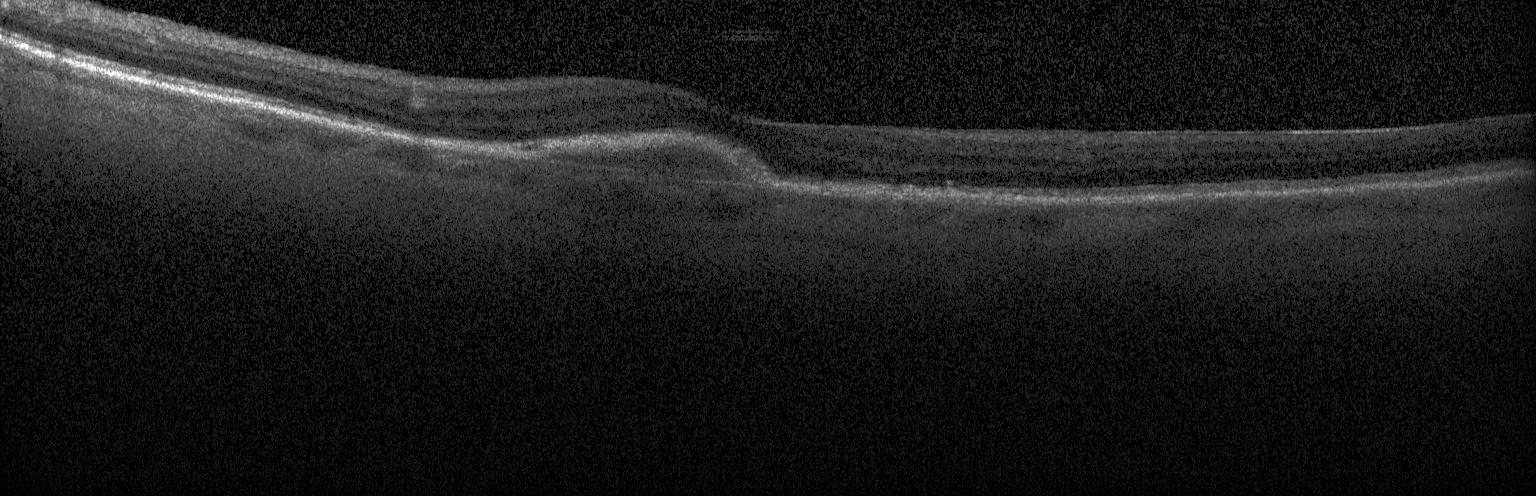
Finding: a choroidal neovascular membrane.